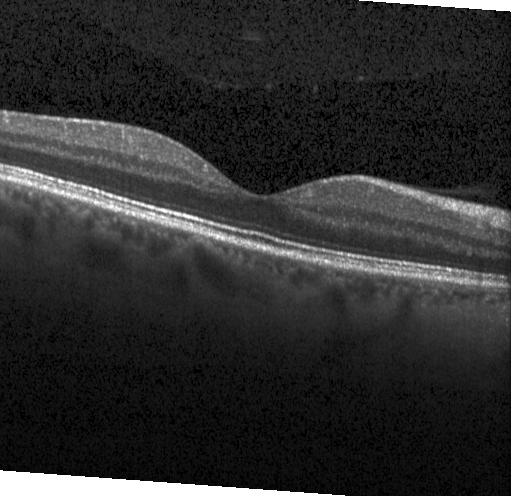

Retinal OCT cross-section; centered on the fovea — Diagnosis: neither choroidal neovascularization, diabetic macular edema, nor drusen.